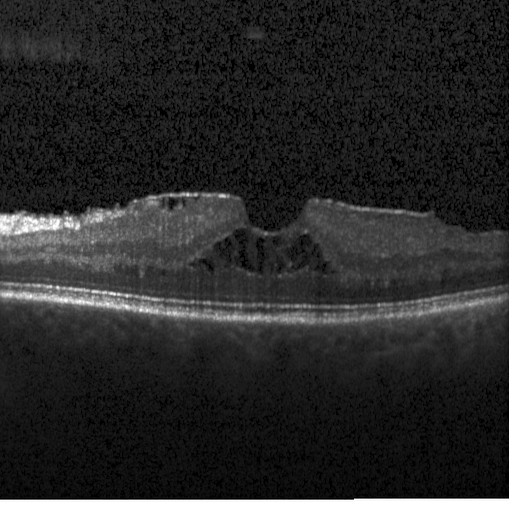
Centered on the fovea, retinal OCT B-scan.
Impression: diabetic macular edema.